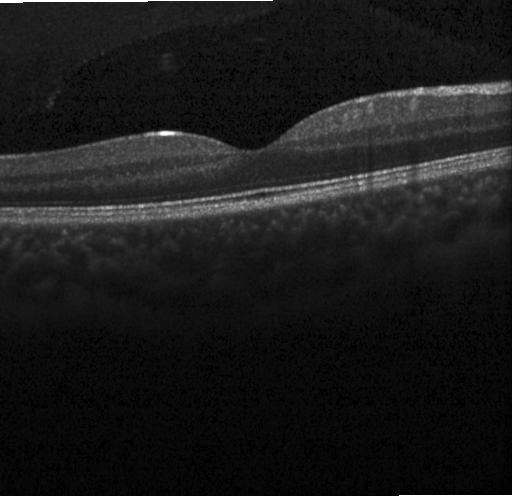

Retinal OCT B-scan; Heidelberg Spectralis; fovea-centered; SD-OCT. The scan shows no CNV, no DME, and no drusen.